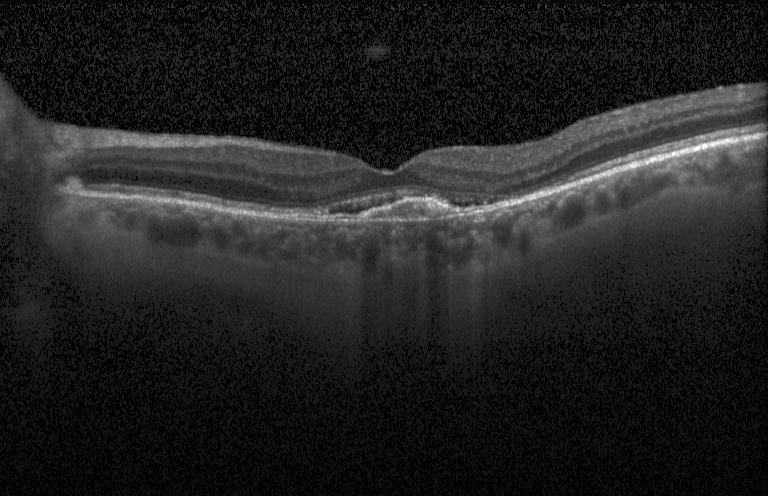 Retinal OCT cross-section showing a choroidal neovascular membrane.